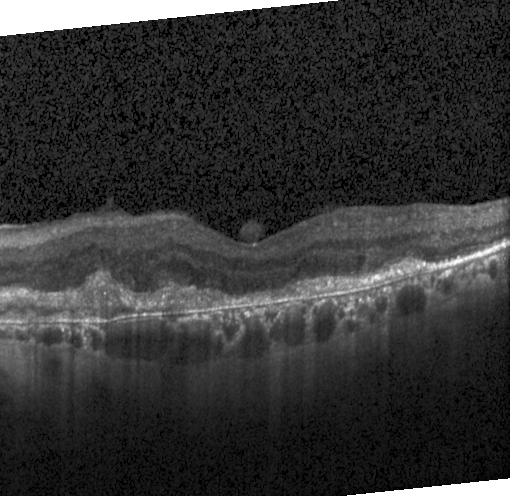
Impression: choroidal neovascularization.